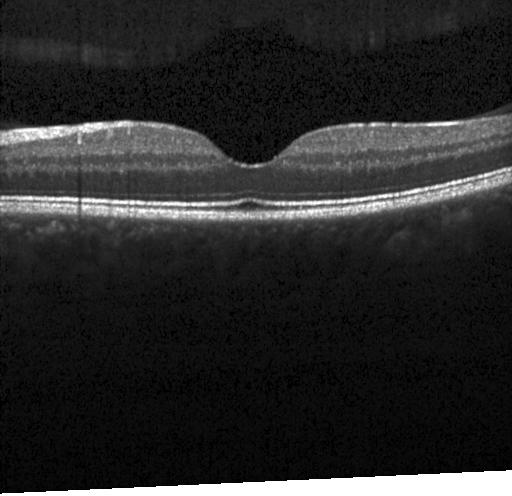

Assessment: no evidence of CNV, DME, or drusen.